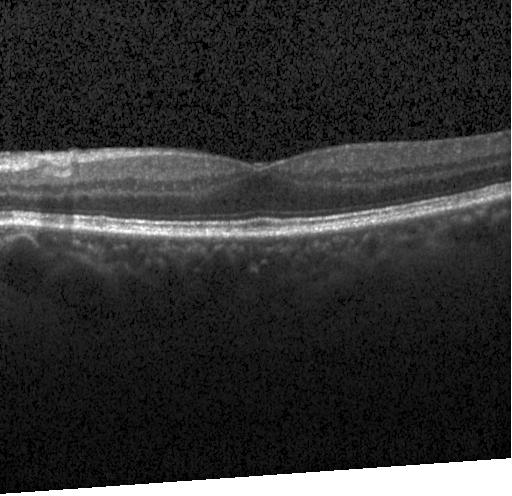 Optical coherence tomography B-scan.
Finding: neither choroidal neovascularization, diabetic macular edema, nor drusen.